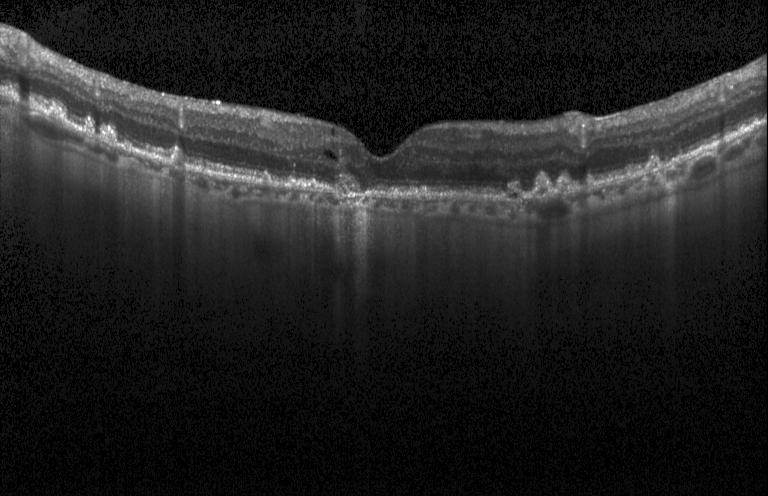
Diagnosis: choroidal neovascularization.